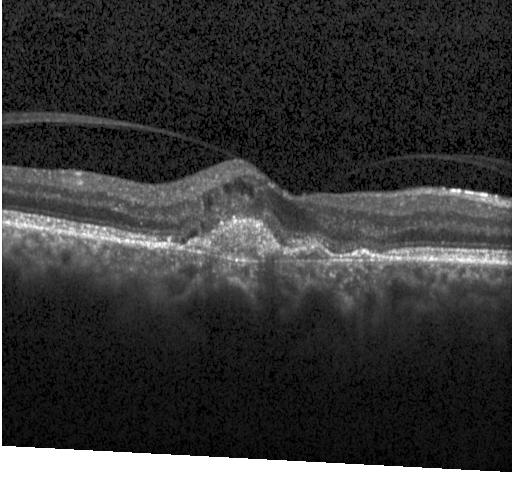

Finding: a choroidal neovascular membrane.